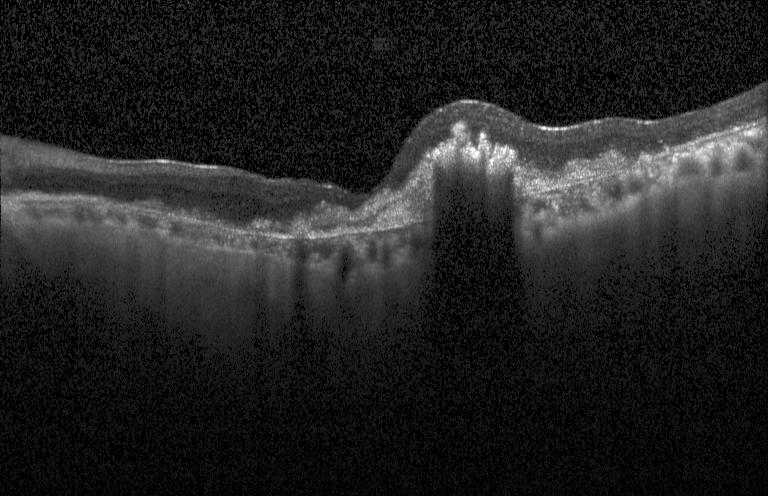

Spectral-domain OCT B-scan: a choroidal neovascular membrane.